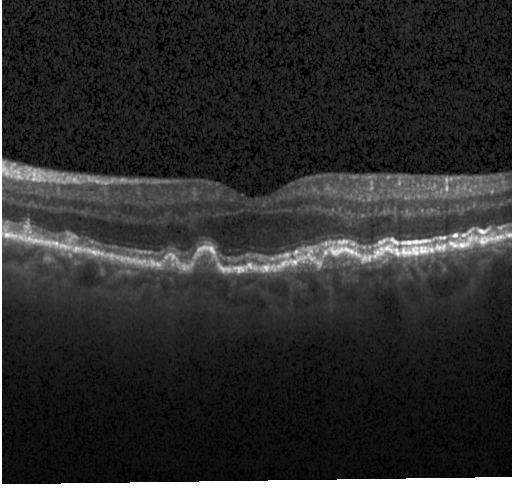

Retinal OCT B-scan
Dx: drusen.